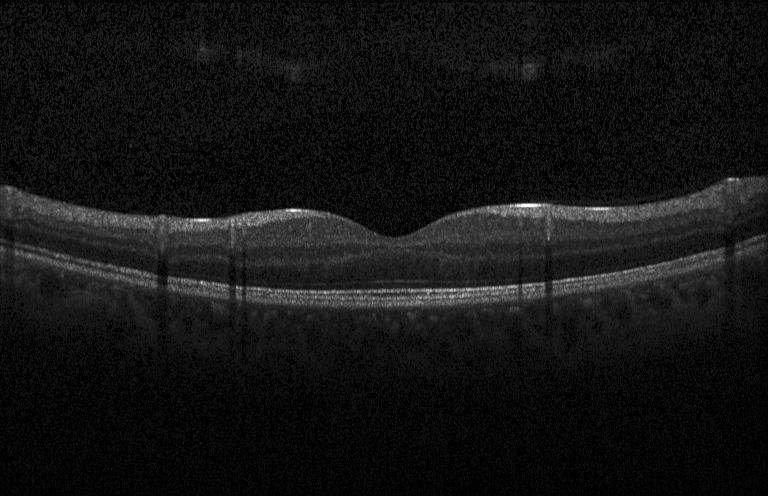 OCT line scan, acquired on a Heidelberg Spectralis.
Diagnosis: neither CNV, DME, nor drusen.